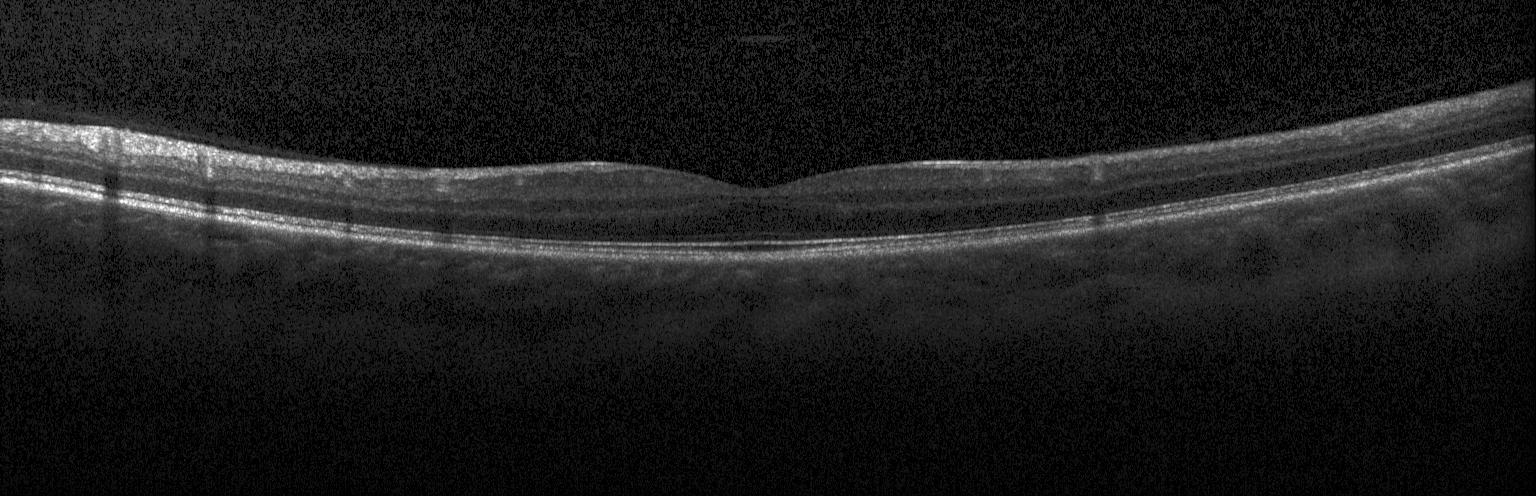
Optical coherence tomography scan
No evidence of choroidal neovascularization, diabetic macular edema, or drusen.